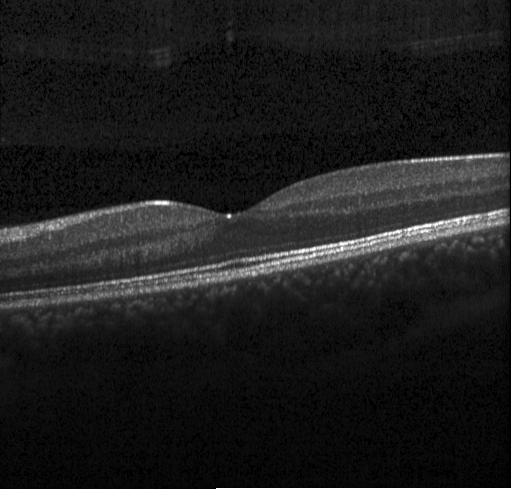

Retinal OCT B-scan. Impression: no evidence of CNV, DME, or drusen.